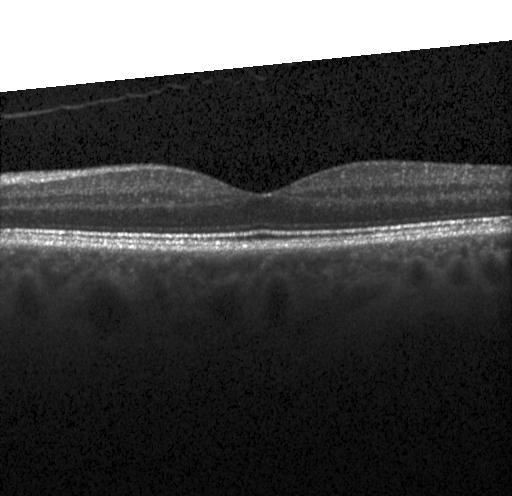
Retinal OCT B-scan
The scan shows neither choroidal neovascularization, diabetic macular edema, nor drusen.